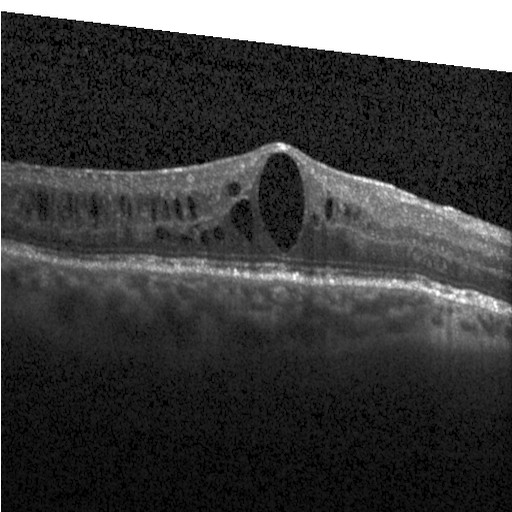

Acquired on a Heidelberg Spectralis, spectral-domain optical coherence tomography, retinal OCT B-scan, horizontal scan through the fovea.
OCT finding: DME.